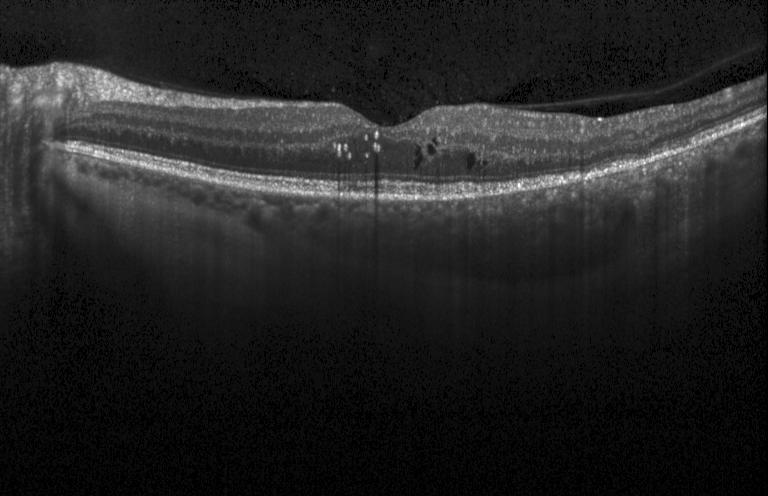 Optical coherence tomography scan, macular scan, SD-OCT, Heidelberg Spectralis OCT system.
Impression: diabetic macular edema.